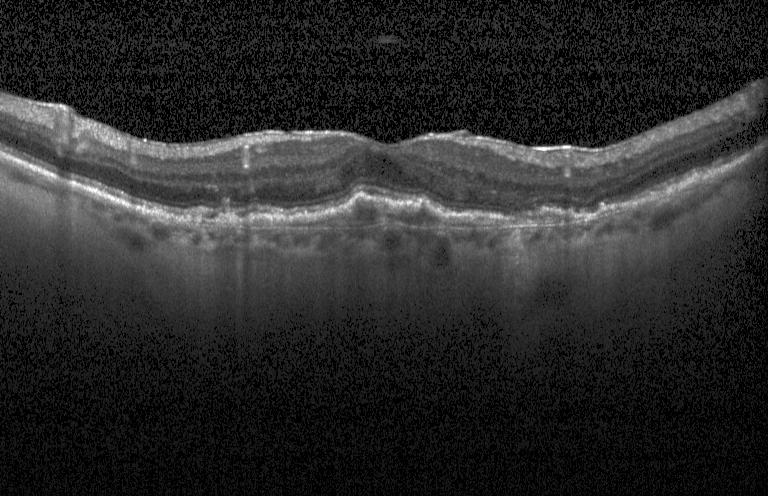
Impression: choroidal neovascularization (CNV).